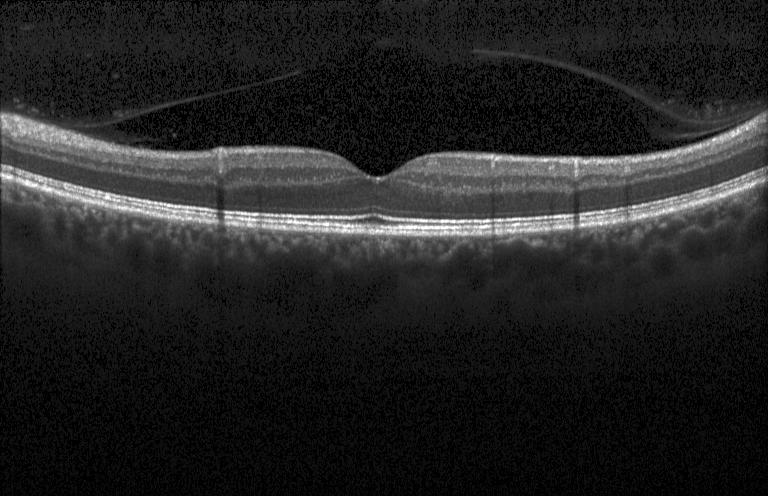

Retinal OCT cross-section.
The scan shows neither choroidal neovascularization, diabetic macular edema, nor drusen.